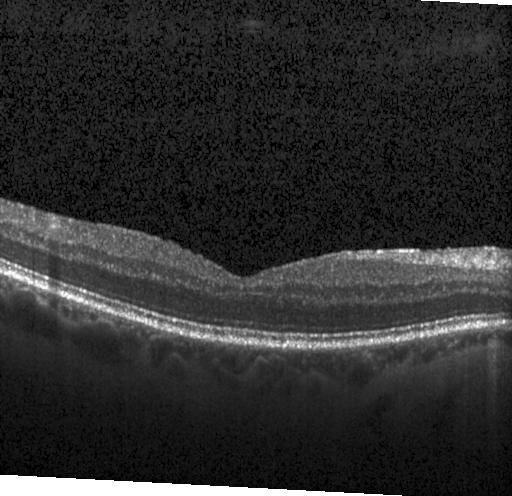

OCT B-scan · SD-OCT.
OCT finding: no choroidal neovascularization, no diabetic macular edema, and no drusen.